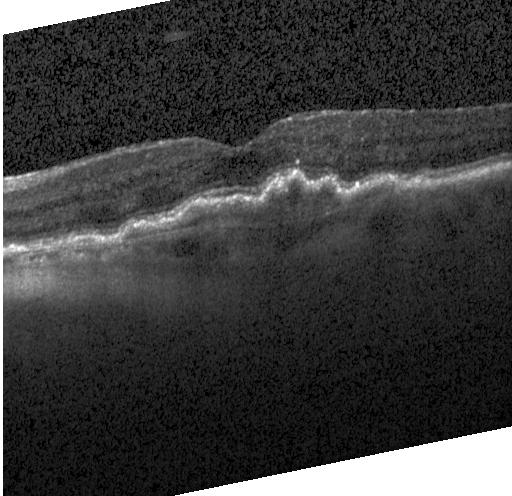
Dx: choroidal neovascularization (CNV).